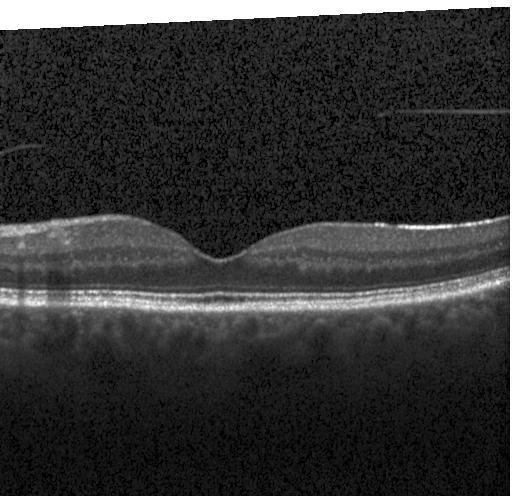 Acquired on a Heidelberg Spectralis · retinal OCT B-scan. Diagnosis: no choroidal neovascularization, diabetic macular edema, or drusen.